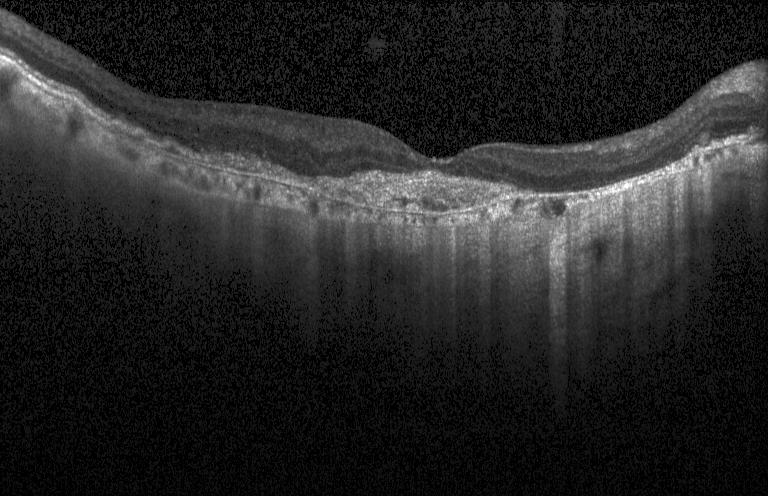 OCT B-scan
Finding: a choroidal neovascular membrane.